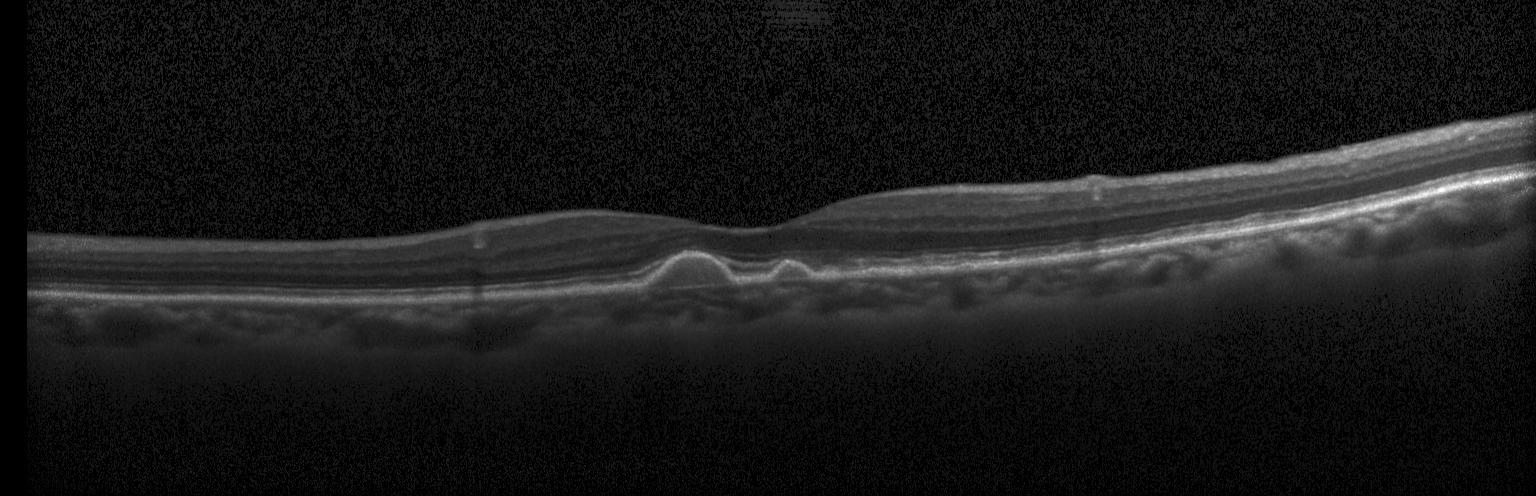 OCT finding: drusen.